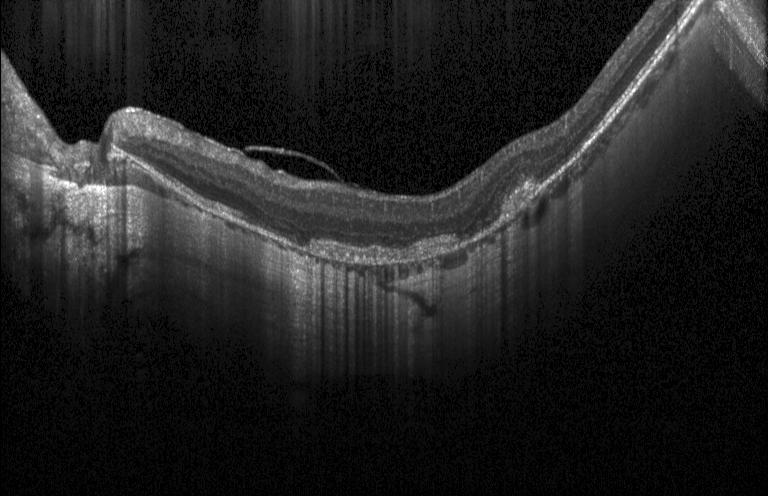 Impression: CNV.